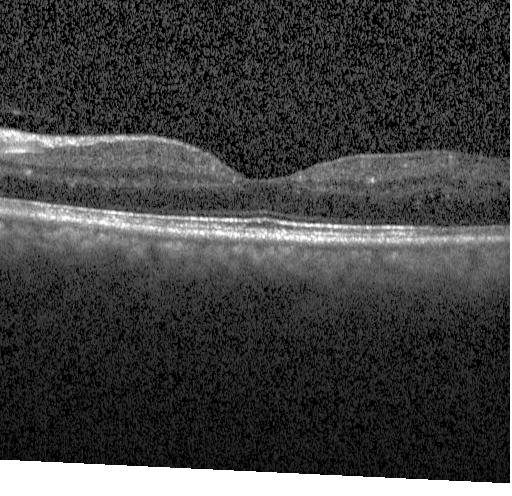

Retinal OCT cross-section.
The scan shows neither choroidal neovascularization, diabetic macular edema, nor drusen.